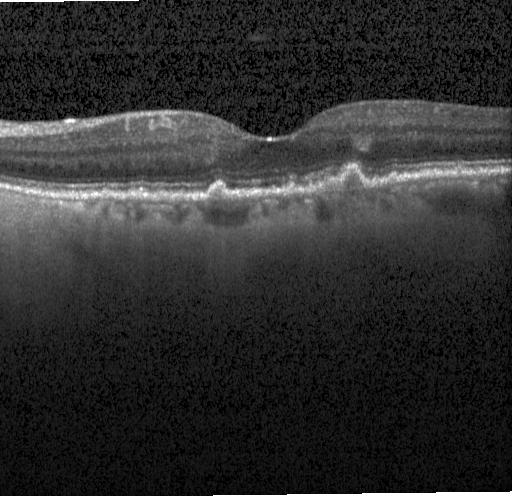 Acquired on a Heidelberg Spectralis. Retinal OCT B-scan. Spectral-domain optical coherence tomography. Through the macula — Finding: drusen.